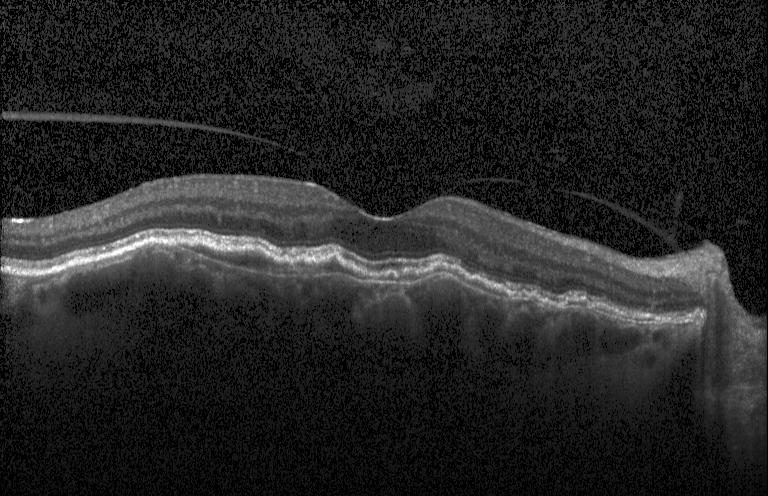
Horizontal scan through the fovea, OCT line scan, Heidelberg Spectralis. Assessment: a choroidal neovascular membrane.